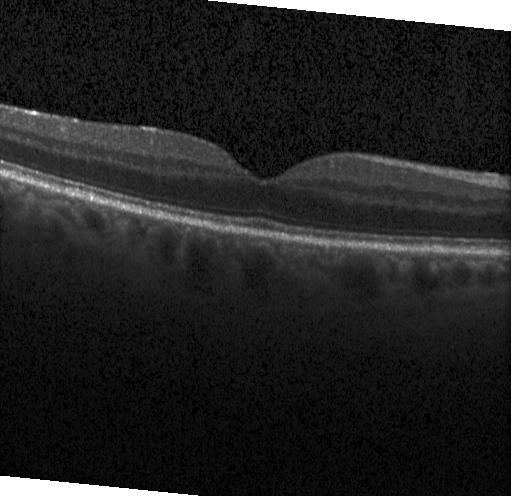 Optical coherence tomography B-scan — The scan shows no CNV, DME, or drusen.